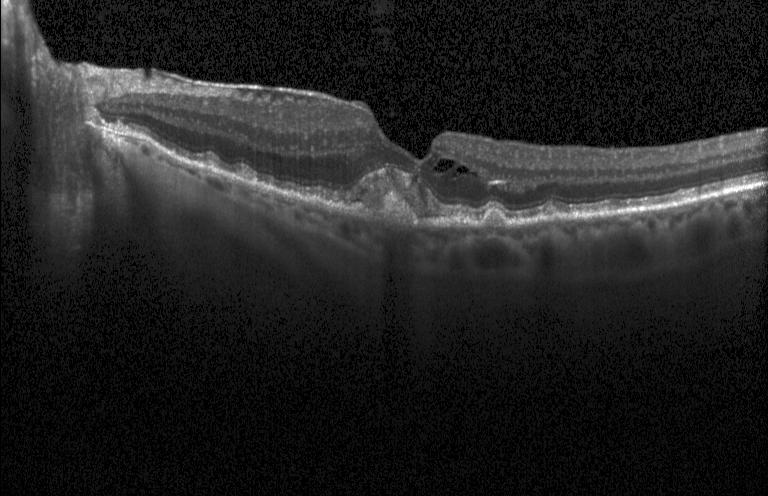
Diagnosis: a choroidal neovascular membrane.